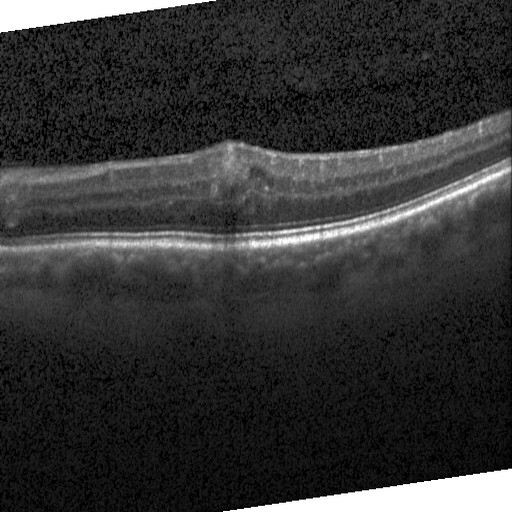 Optical coherence tomography scan, acquired on a Heidelberg Spectralis — Macular OCT: diabetic macular edema.